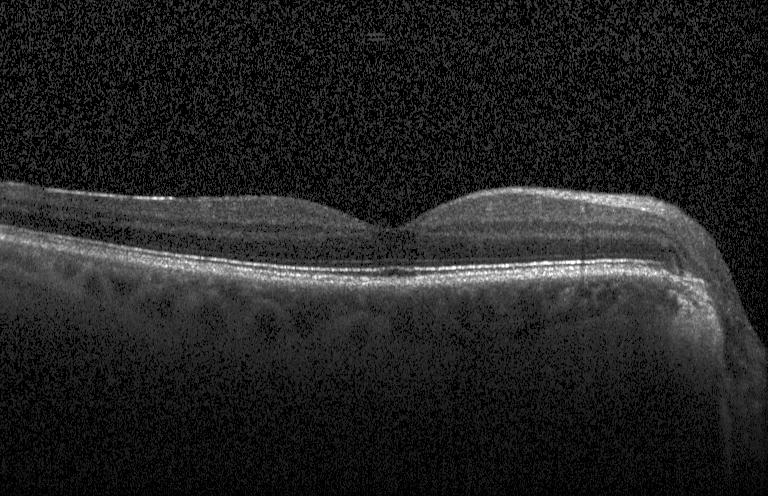

Dx: no choroidal neovascularization, no diabetic macular edema, and no drusen.